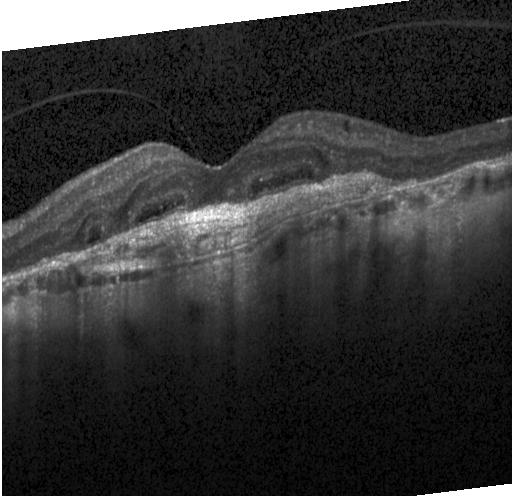 Through the macula; spectral-domain optical coherence tomography; Heidelberg Spectralis OCT system; OCT B-scan.
Dx: CNV.